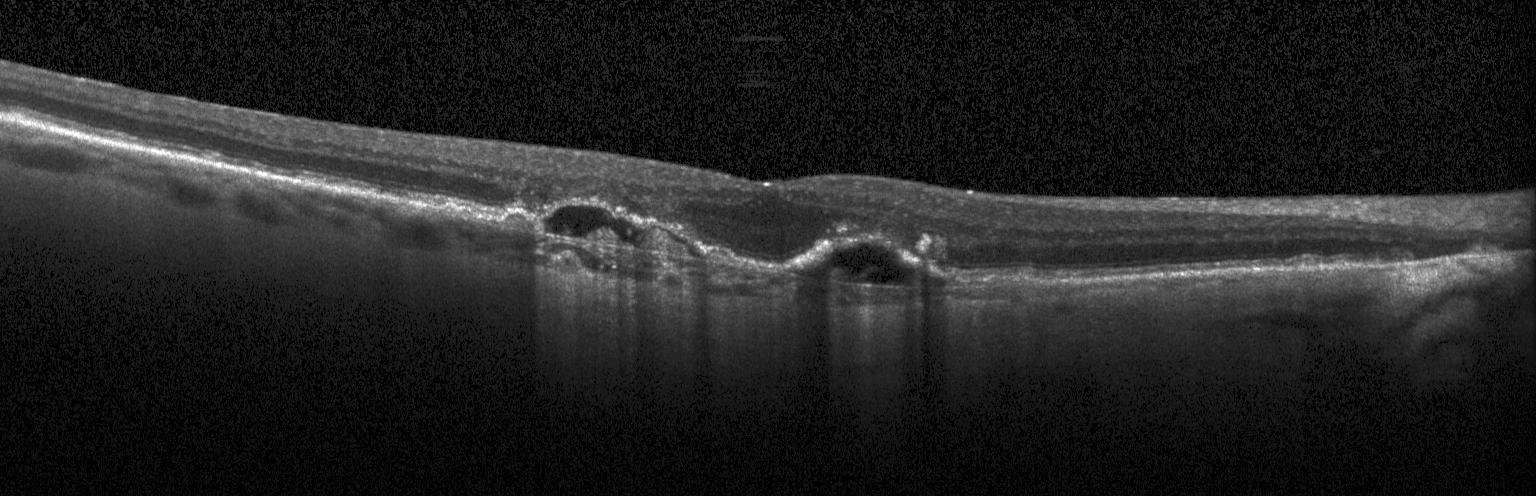 Spectral-domain OCT B-scan: choroidal neovascularization.